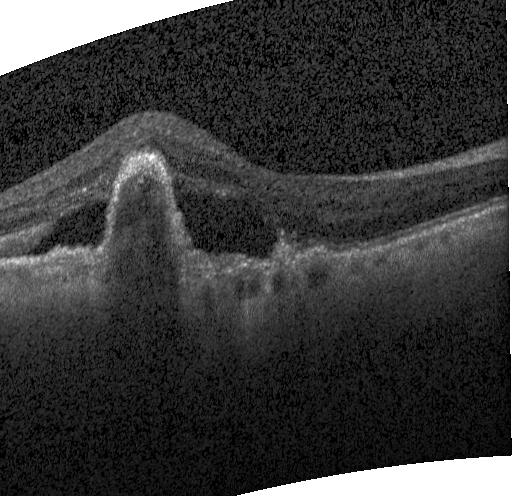
OCT line scan
Diagnosis: choroidal neovascularization.